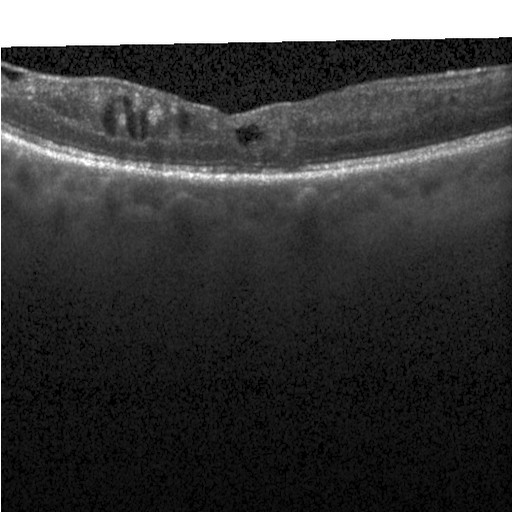
Impression: DME.